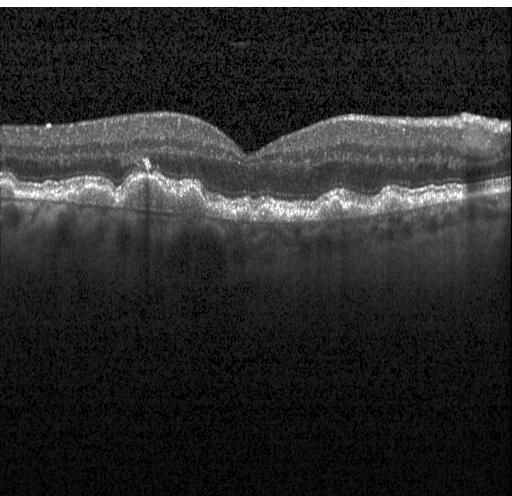 Retinal OCT cross-section · fovea-centered · spectral-domain OCT · Heidelberg Spectralis. The scan shows multiple drusen.